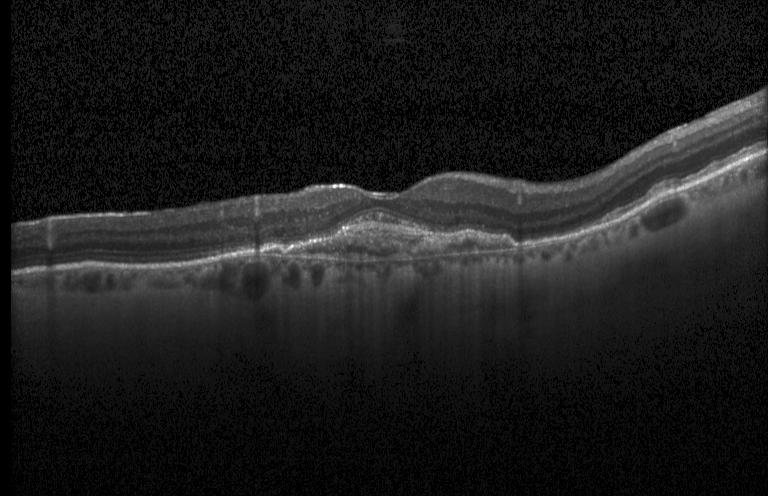
OCT line scan.
The scan shows a choroidal neovascular membrane.